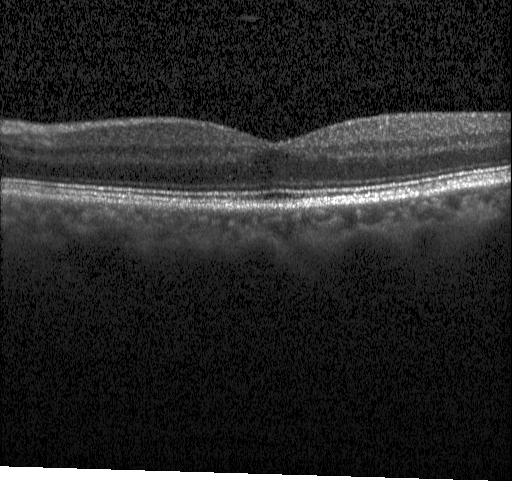 Acquired on a Heidelberg Spectralis · SD-OCT · OCT B-scan · horizontal scan through the fovea.
This B-scan demonstrates neither choroidal neovascularization, diabetic macular edema, nor drusen.